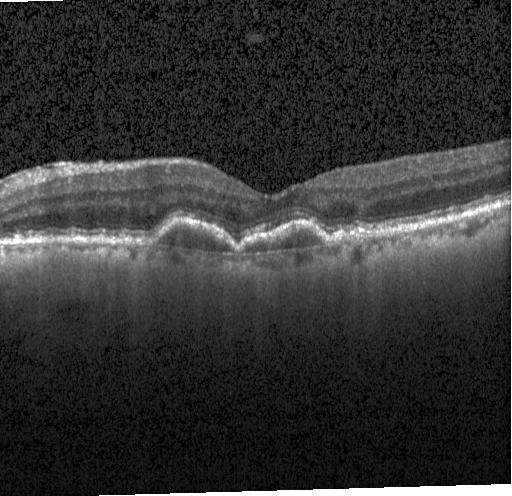

Retinal OCT B-scan. Centered on the fovea.
The scan shows choroidal neovascularization (CNV).